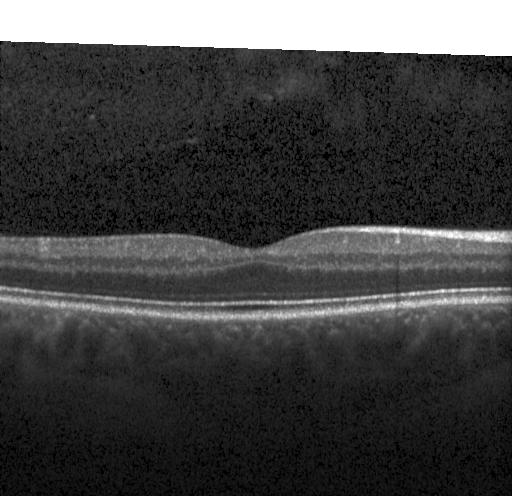
OCT B-scan. Impression: no choroidal neovascularization, diabetic macular edema, or drusen.